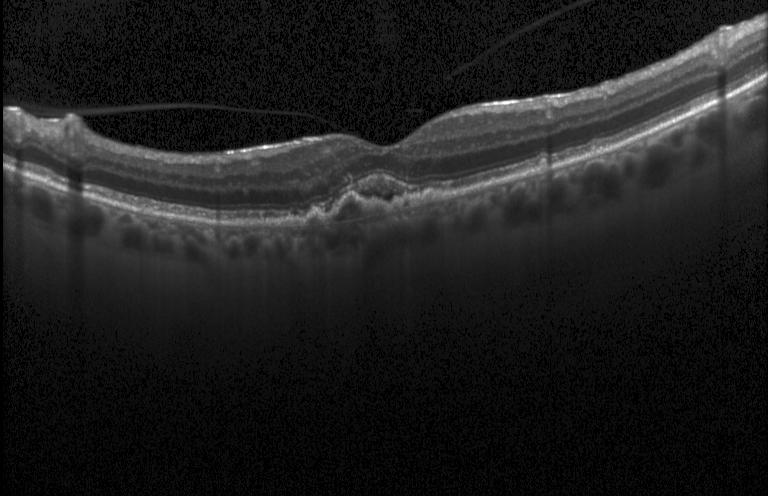
OCT line scan, spectral-domain OCT
Diagnosis: CNV.